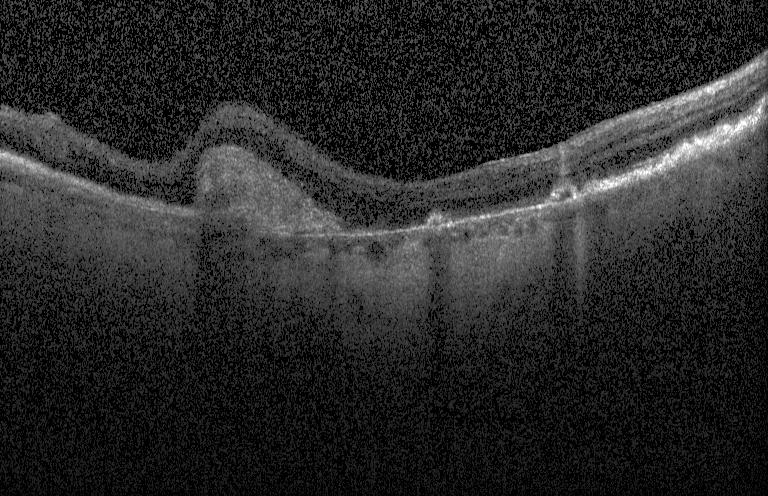 Spectral-domain optical coherence tomography, horizontal scan through the fovea, OCT B-scan, Heidelberg Spectralis.
The scan shows a choroidal neovascular membrane.